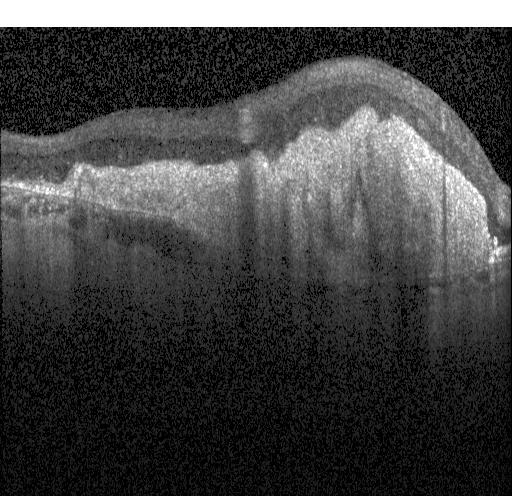

Horizontal scan through the fovea. Retinal OCT cross-section
Dx: choroidal neovascularization.